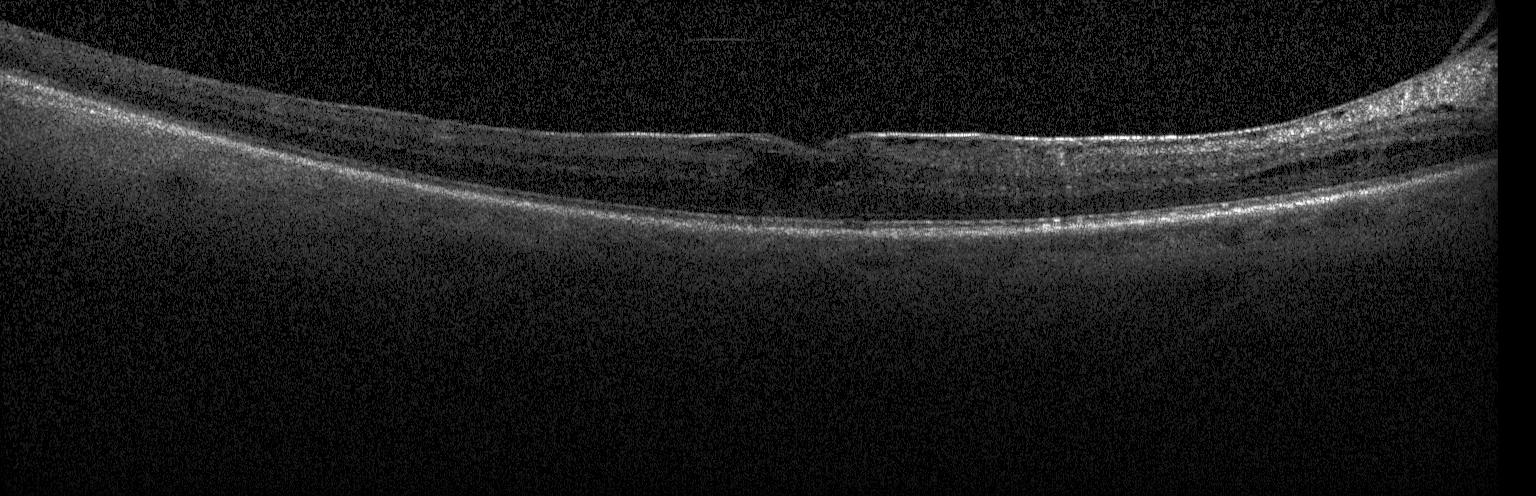 OCT scan showing diabetic macular edema (DME).